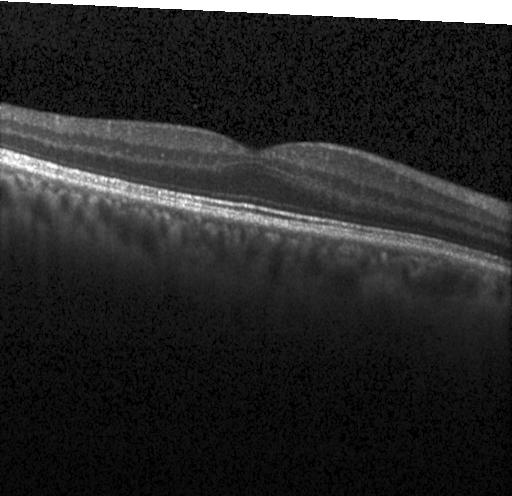

Retinal OCT cross-section showing no CNV, no DME, and no drusen.